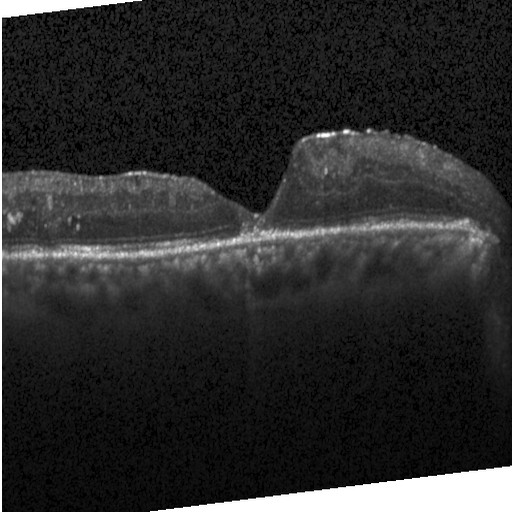 Macular OCT: diabetic macular edema (DME).